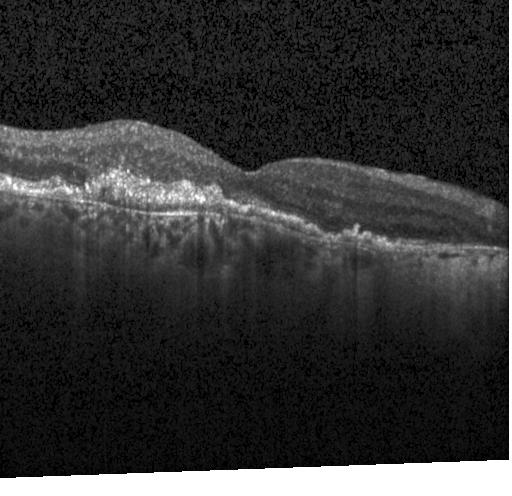
OCT line scan; SD-OCT; centered on the fovea; Heidelberg Spectralis OCT system. Impression: choroidal neovascularization.